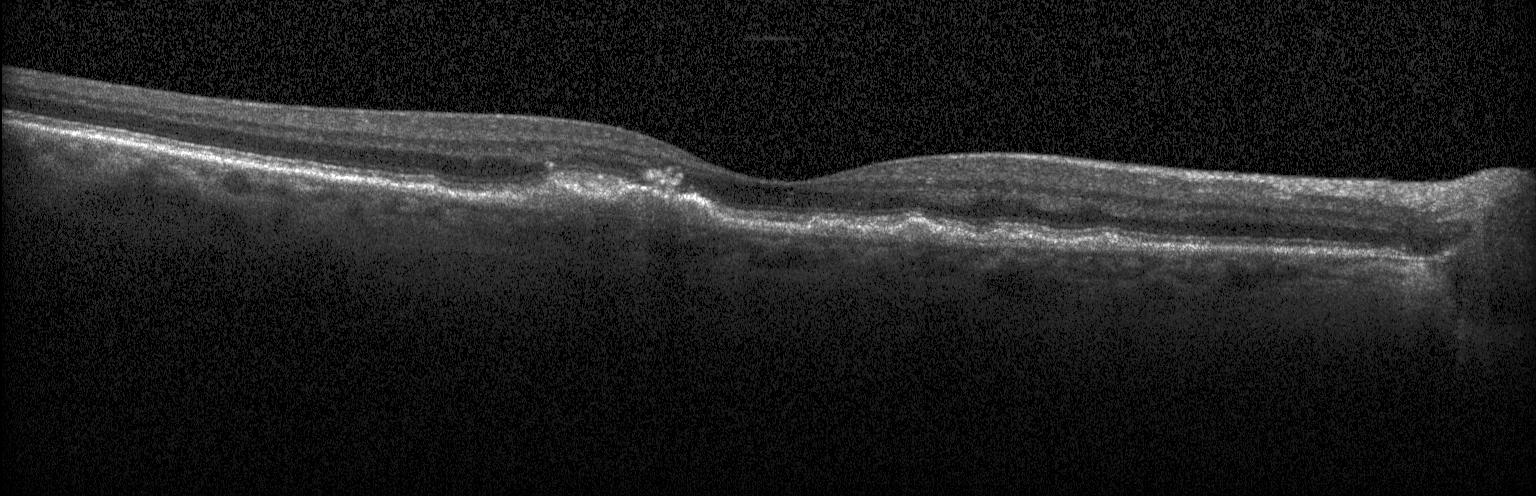
Dx: a choroidal neovascular membrane.